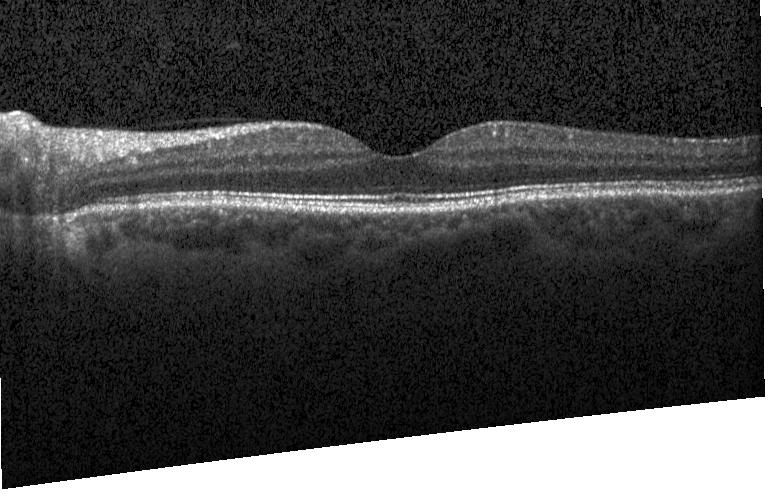 Heidelberg Spectralis, optical coherence tomography B-scan, macular scan. Finding: no evidence of choroidal neovascularization, diabetic macular edema, or drusen.